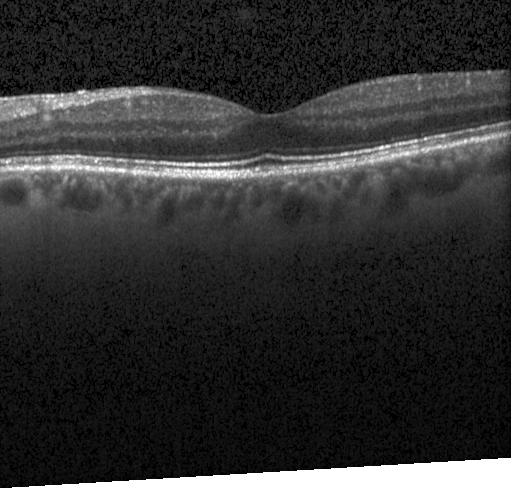
SD-OCT; optical coherence tomography B-scan
Finding: neither CNV, DME, nor drusen.